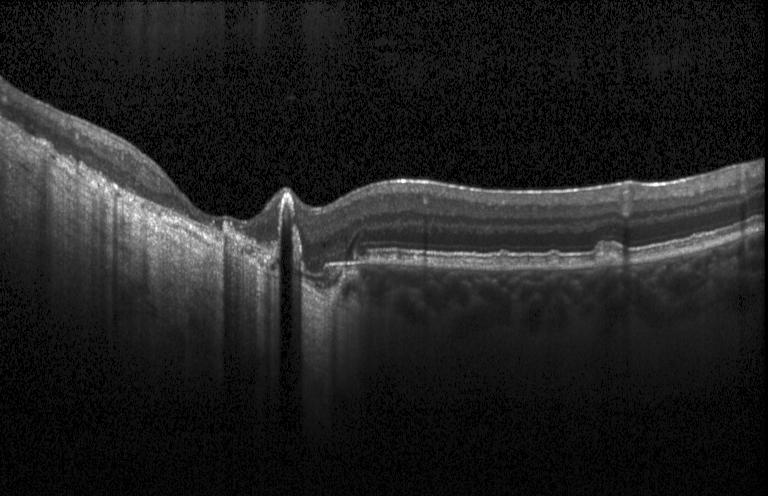
OCT B-scan, through the macula, spectral-domain optical coherence tomography, instrument: Heidelberg Spectralis
Diagnosis: a choroidal neovascular membrane.